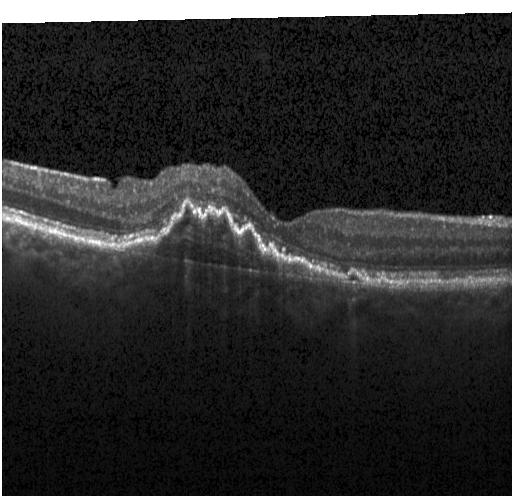
Assessment: a choroidal neovascular membrane.